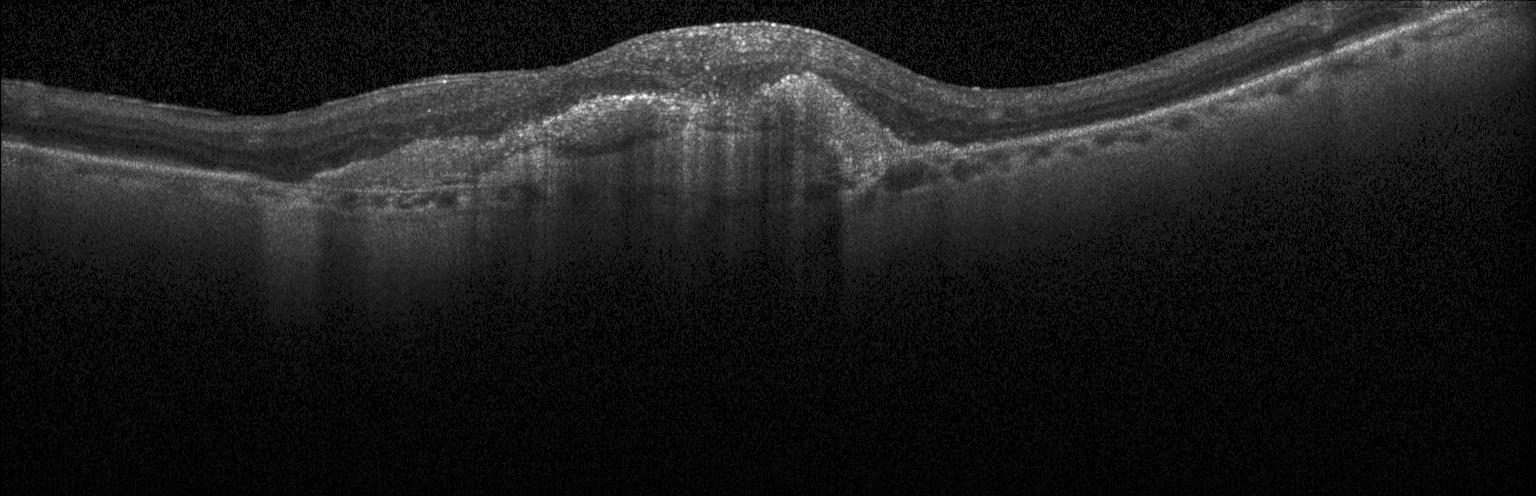
Retinal OCT cross-section showing CNV.